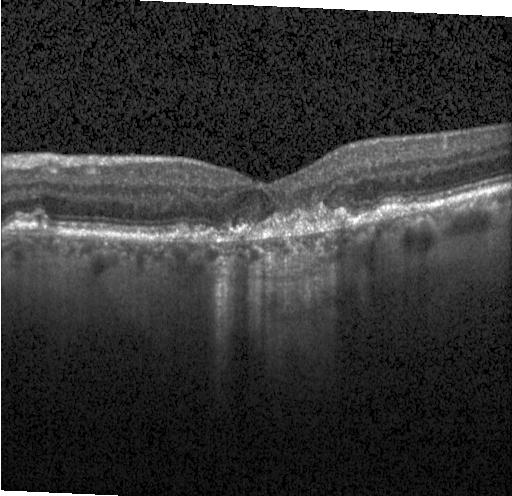
Spectral-domain optical coherence tomography; centered on the fovea; retinal OCT cross-section.
OCT finding: choroidal neovascularization.